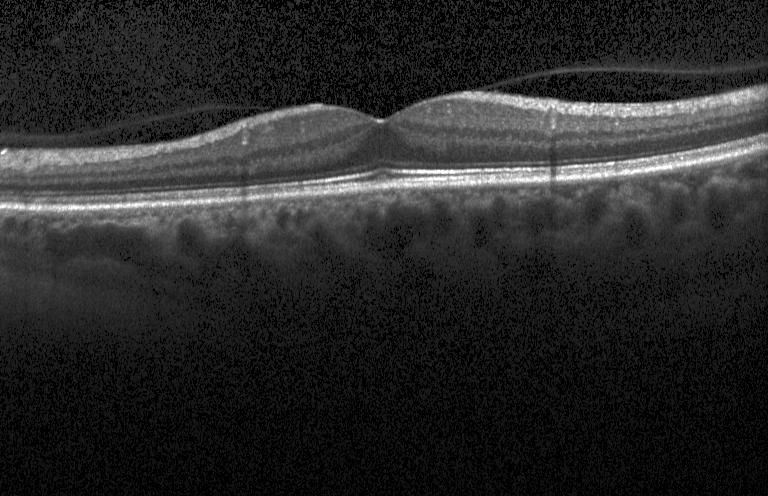
Retinal OCT B-scan.
Diagnosis: neither choroidal neovascularization, diabetic macular edema, nor drusen.